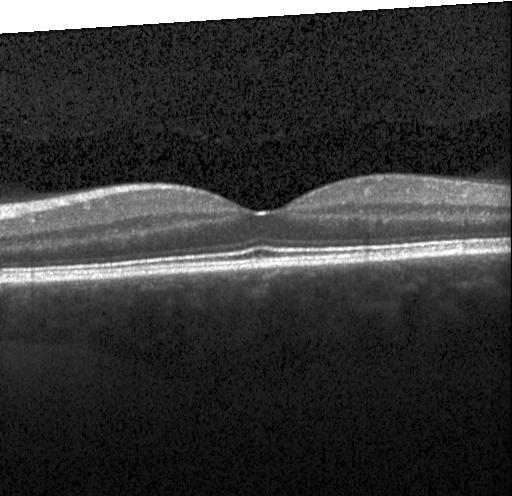

Through the macula, instrument: Heidelberg Spectralis, spectral-domain optical coherence tomography, OCT B-scan
Neither choroidal neovascularization, diabetic macular edema, nor drusen.